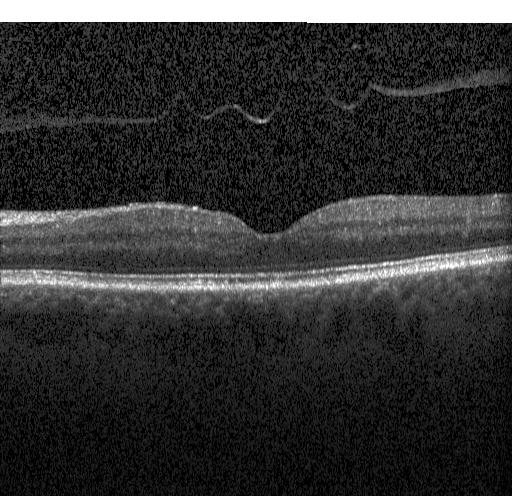

Acquired on a Heidelberg Spectralis, SD-OCT, optical coherence tomography scan, centered on the fovea — Diagnosis: no CNV, DME, or drusen.